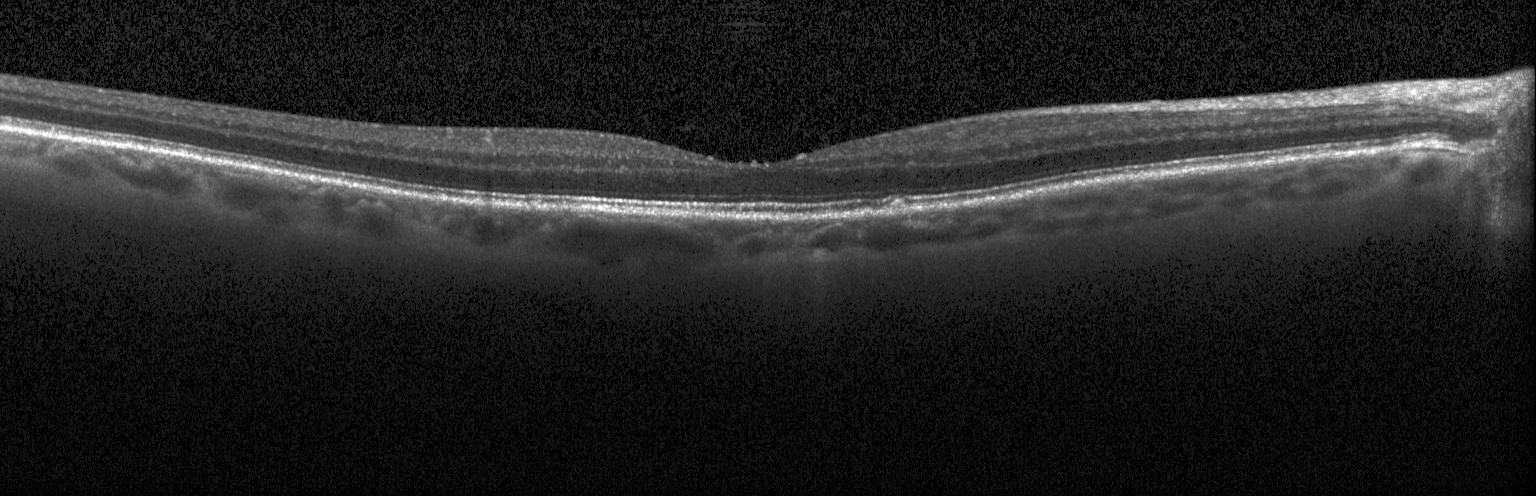

Spectral-domain OCT; optical coherence tomography B-scan. Diagnosis: drusen.